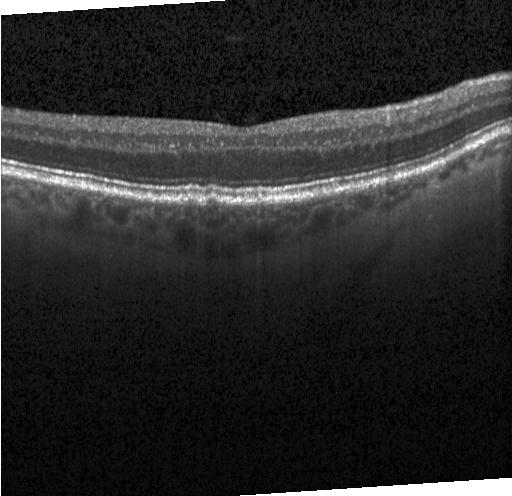 OCT line scan · Heidelberg Spectralis OCT system
Macular OCT: sub-RPE drusenoid deposits.